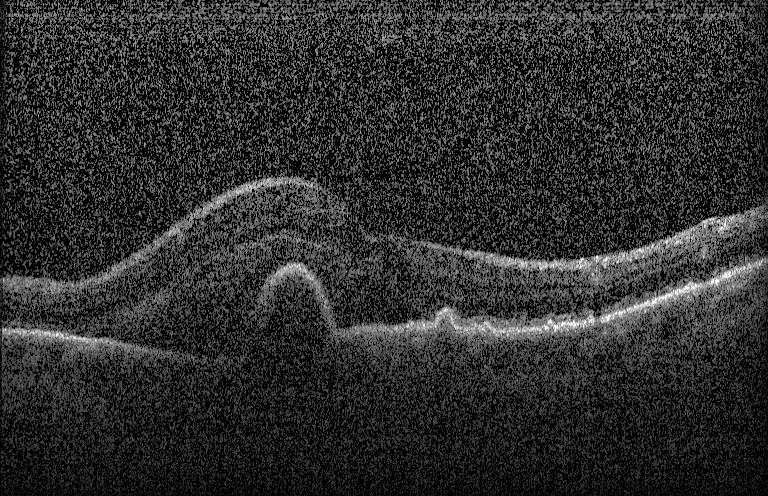 OCT B-scan. Finding: choroidal neovascularization.